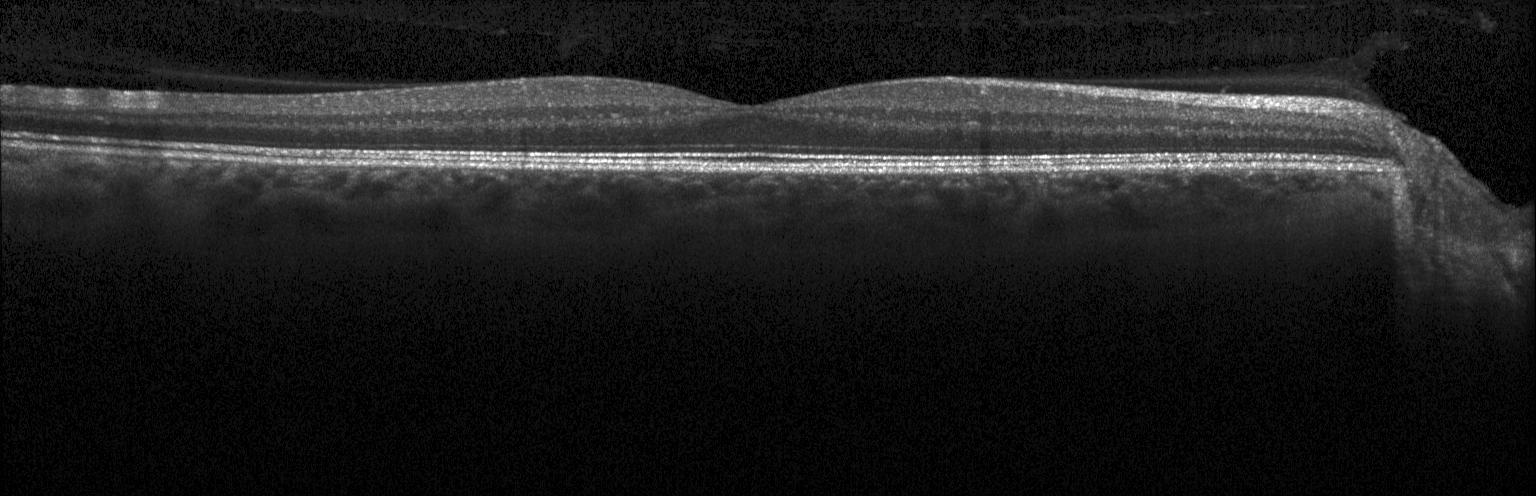 Spectral-domain optical coherence tomography; optical coherence tomography B-scan.
Finding: no CNV, DME, or drusen.